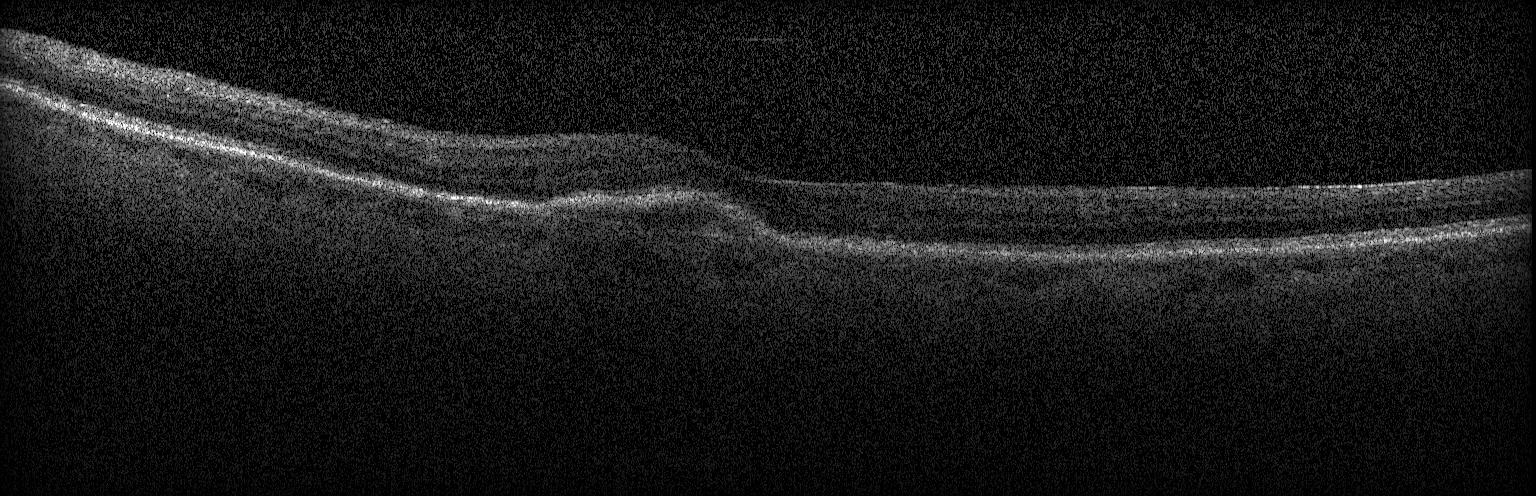

OCT B-scan. Diagnosis: a choroidal neovascular membrane.